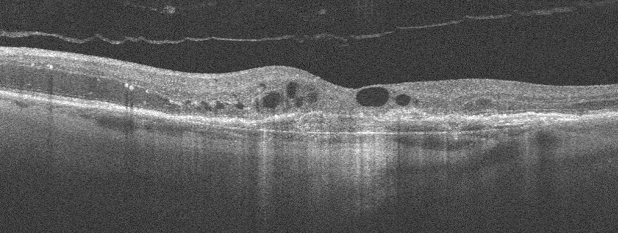 Right eye · retinal OCT cross-section.
Diagnosis: AMD.